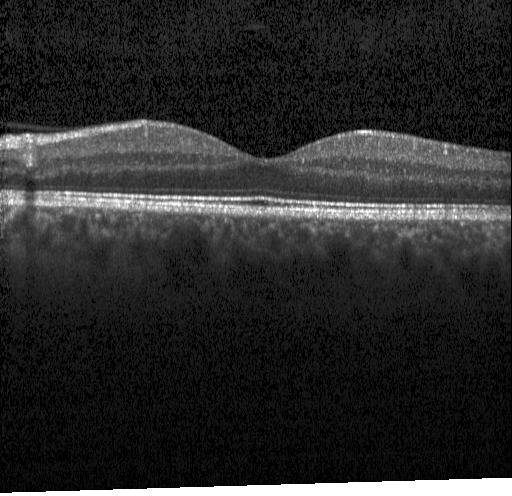 OCT line scan.
Dx: no evidence of choroidal neovascularization, diabetic macular edema, or drusen.